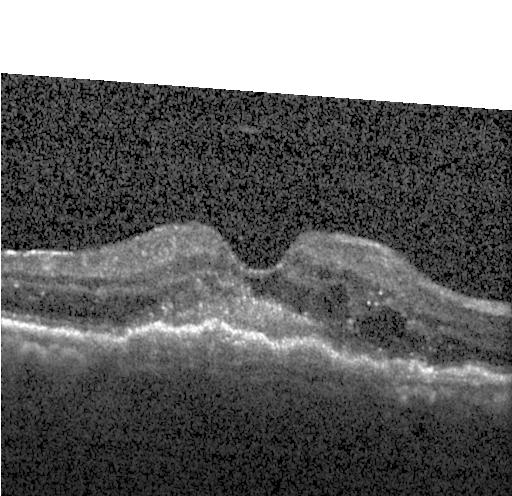 SD-OCT · acquired on a Heidelberg Spectralis · OCT line scan · horizontal scan through the fovea. Finding: a choroidal neovascular membrane.